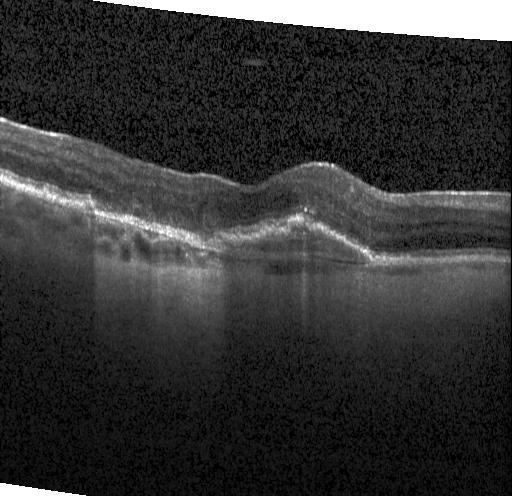

Fovea-centered. Heidelberg Spectralis. Spectral-domain optical coherence tomography. OCT B-scan. Impression: a choroidal neovascular membrane.